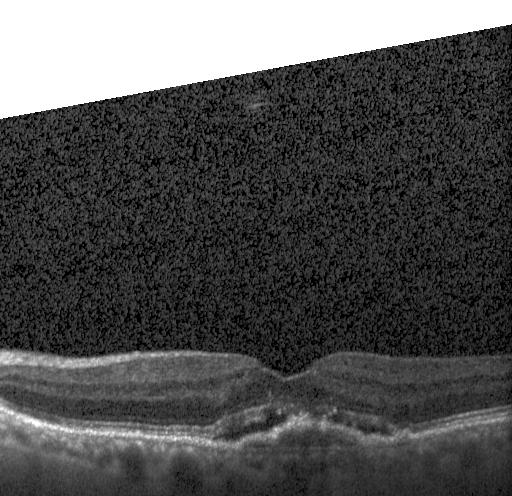
Horizontal scan through the fovea · instrument: Heidelberg Spectralis · optical coherence tomography B-scan — OCT finding: a choroidal neovascular membrane.